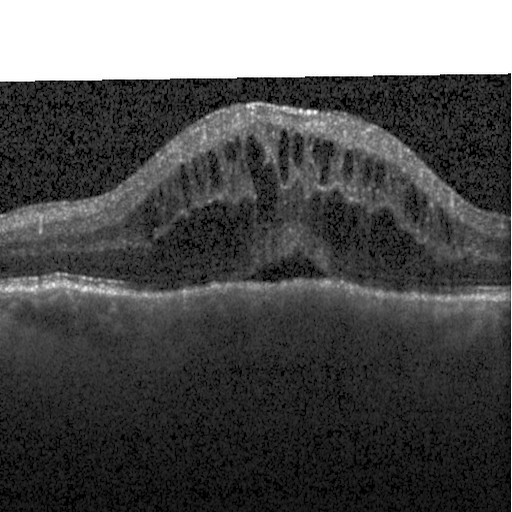
Retinal OCT cross-section showing diabetic macular edema.